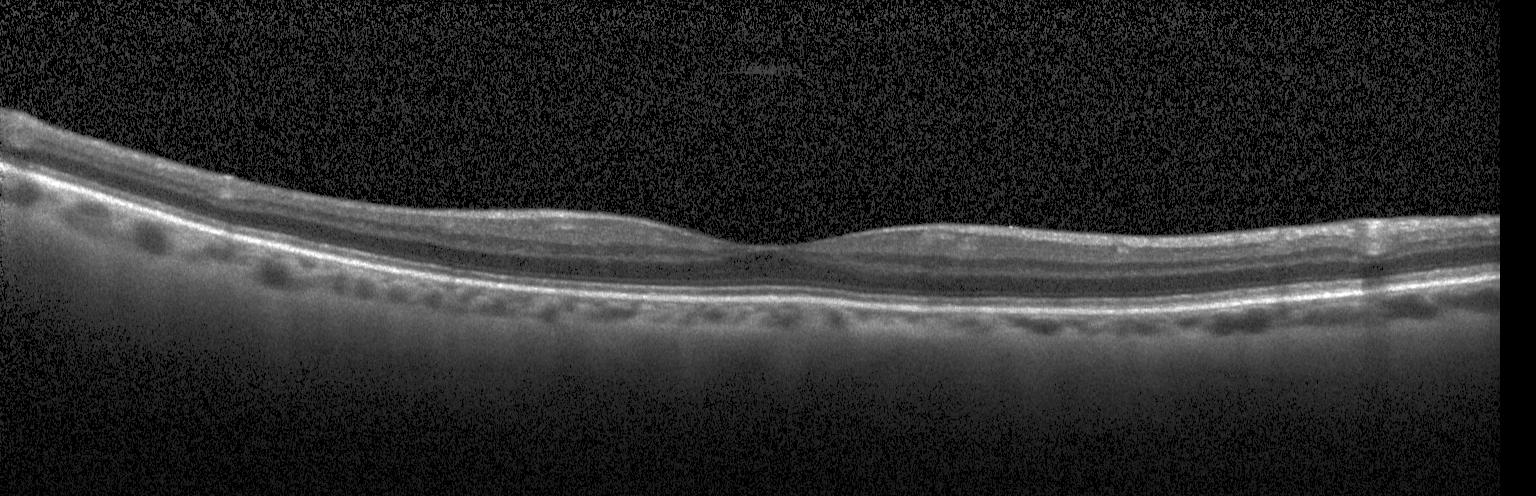 Horizontal scan through the fovea, spectral-domain OCT, retinal OCT B-scan. Impression: no choroidal neovascularization, no diabetic macular edema, and no drusen.